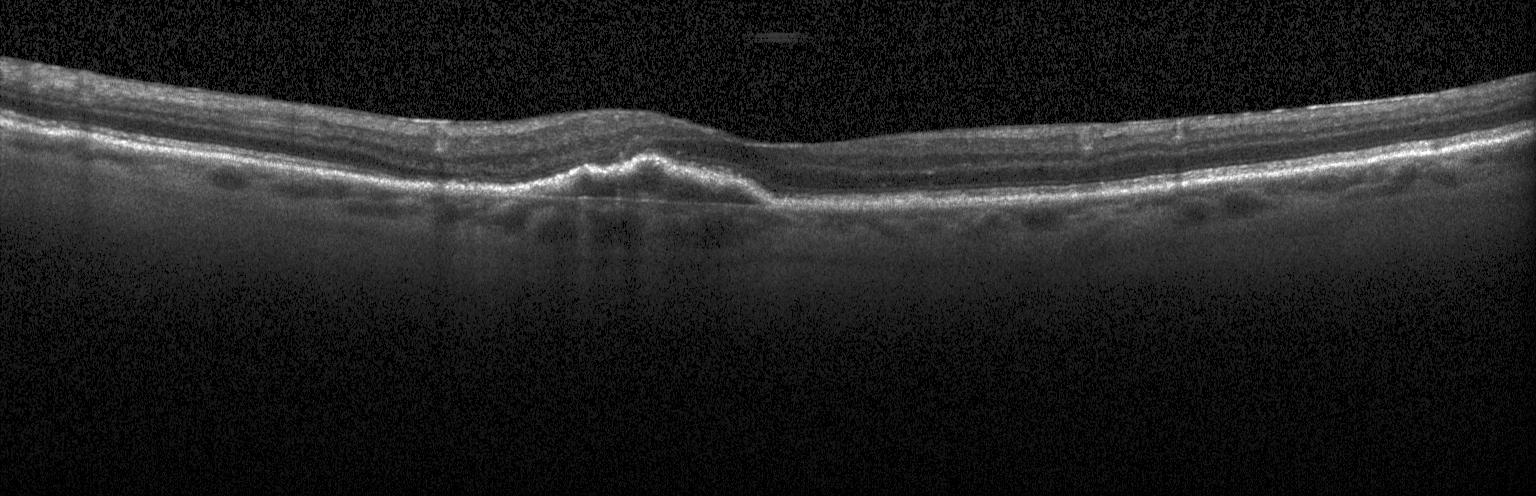

Heidelberg Spectralis OCT system · optical coherence tomography B-scan.
Choroidal neovascularization (CNV).